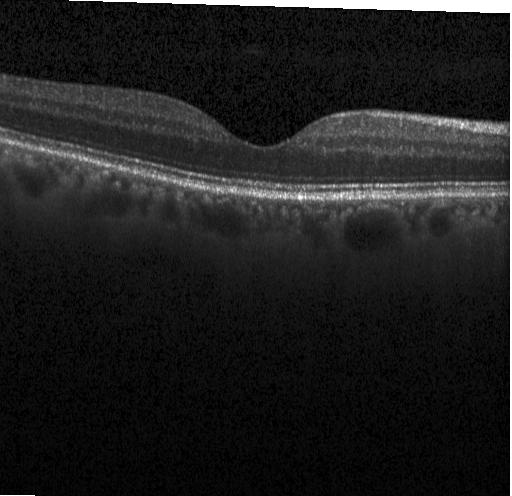

Impression: neither choroidal neovascularization, diabetic macular edema, nor drusen.